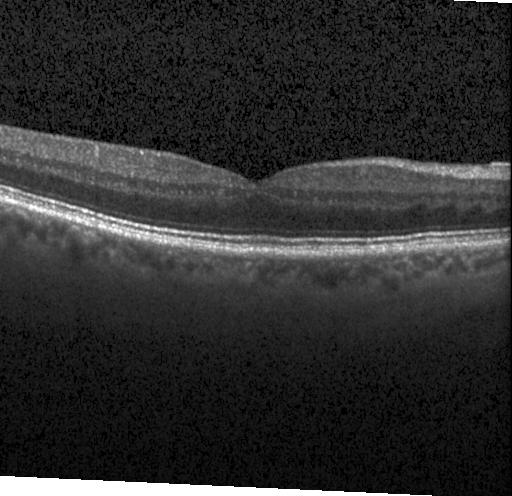

Macular OCT: no evidence of CNV, DME, or drusen.